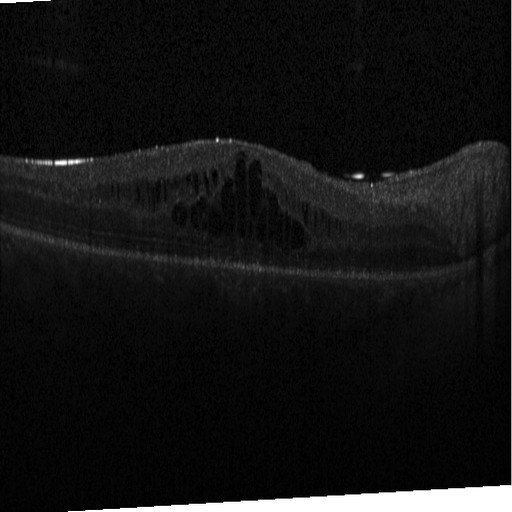
Optical coherence tomography scan, horizontal scan through the fovea. Impression: diabetic macular edema.